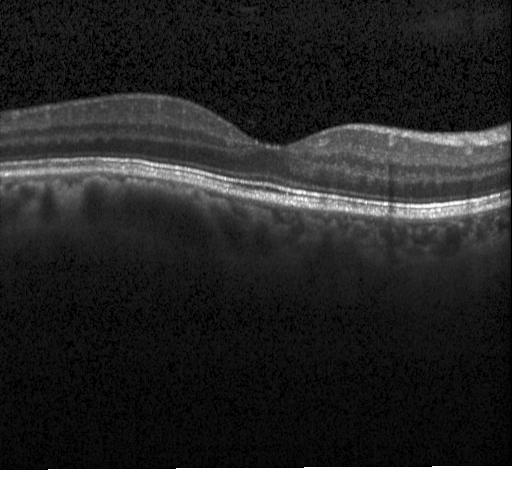

Assessment: no choroidal neovascularization, no diabetic macular edema, and no drusen.